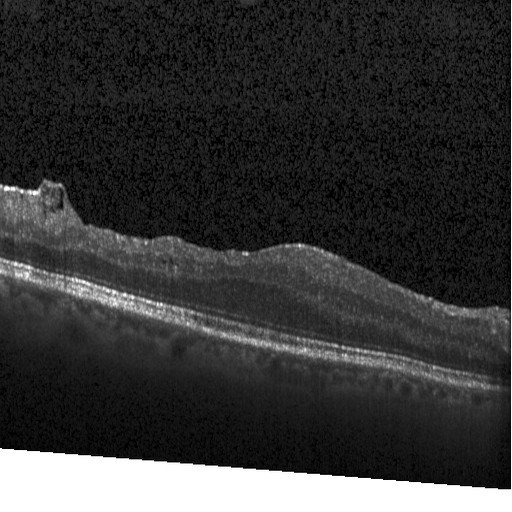
Spectral-domain OCT, optical coherence tomography scan — Diabetic macular edema.